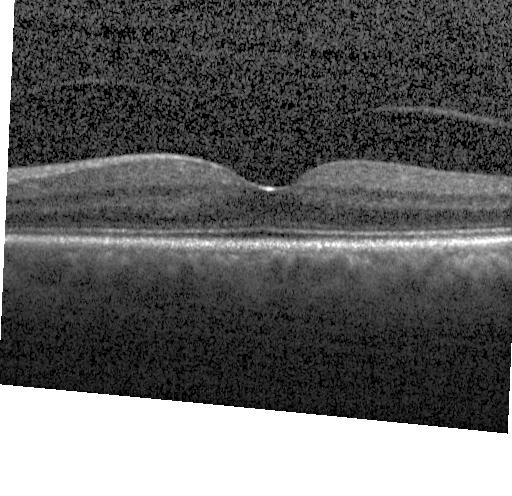 This B-scan demonstrates neither choroidal neovascularization, diabetic macular edema, nor drusen.